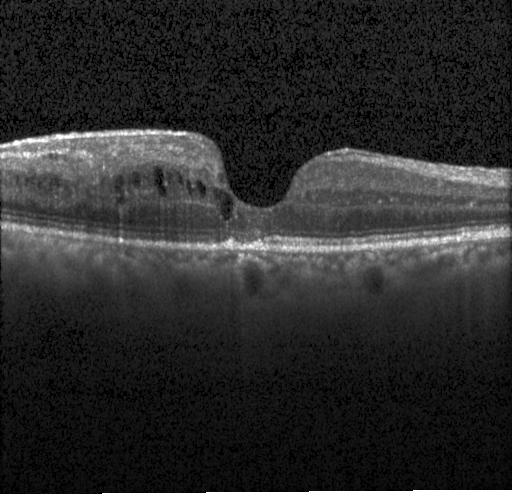
Dx: diabetic macular edema.